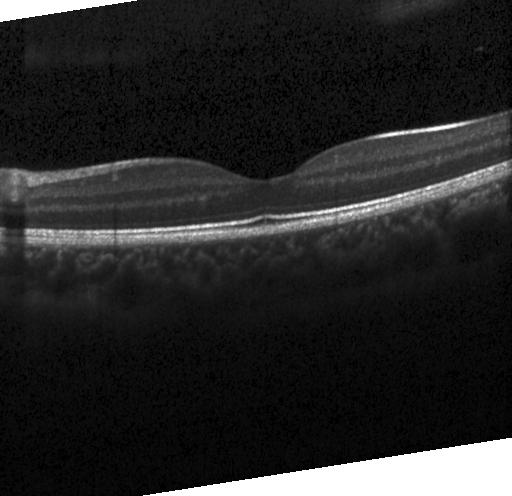
Assessment: no CNV, no DME, and no drusen.